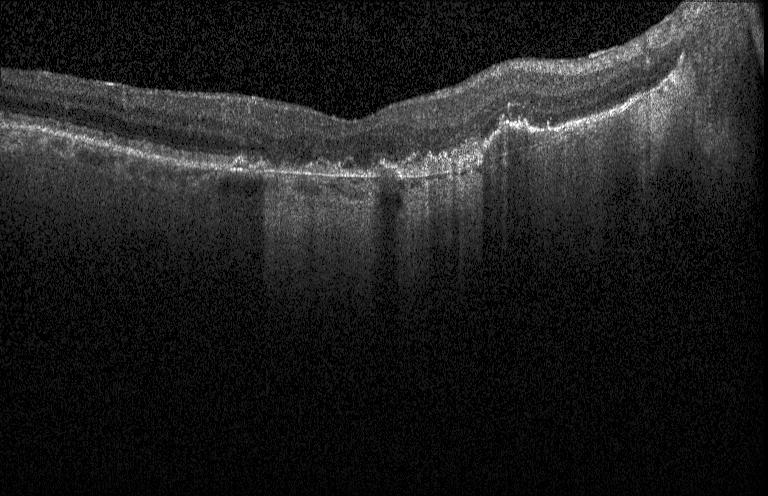
Impression: choroidal neovascularization (CNV).